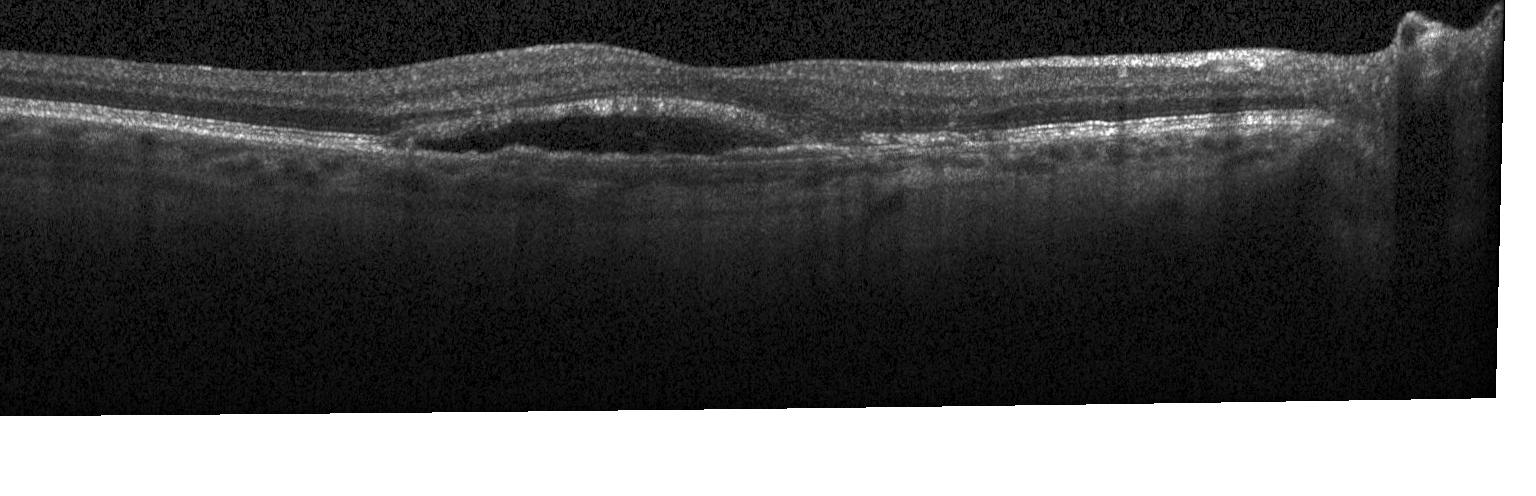
Spectral-domain optical coherence tomography. Heidelberg Spectralis. Horizontal scan through the fovea. Optical coherence tomography scan — Diagnosis: choroidal neovascularization.